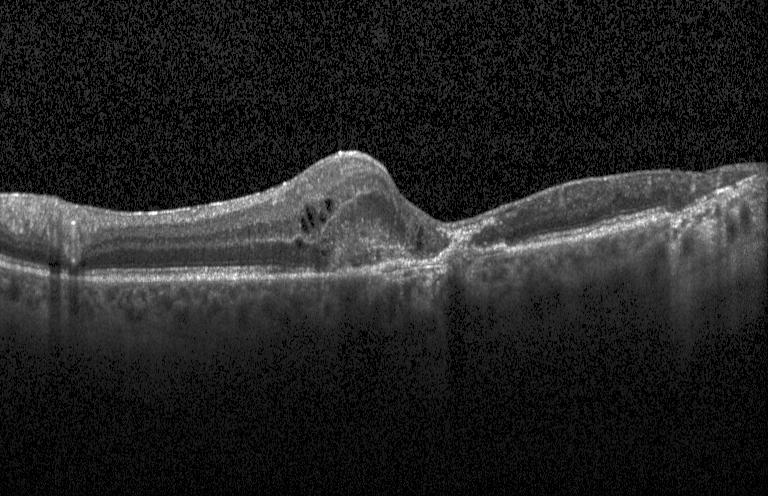 Macular OCT demonstrating choroidal neovascularization (CNV).